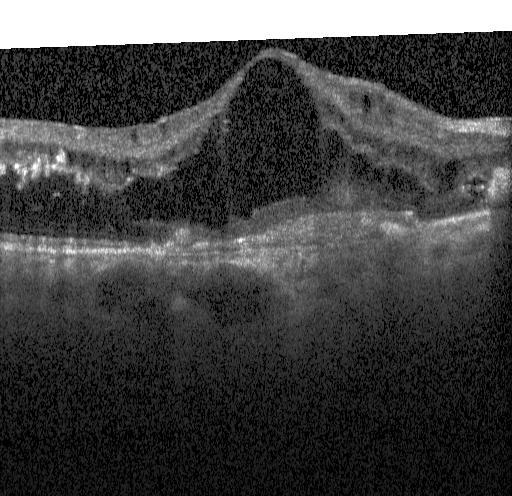 OCT scan showing a choroidal neovascular membrane.